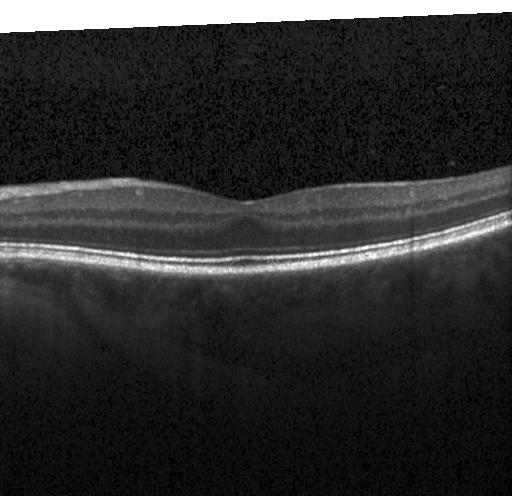

Heidelberg Spectralis OCT system. Spectral-domain optical coherence tomography. Retinal OCT cross-section. Centered on the fovea.
Impression: no CNV, DME, or drusen.